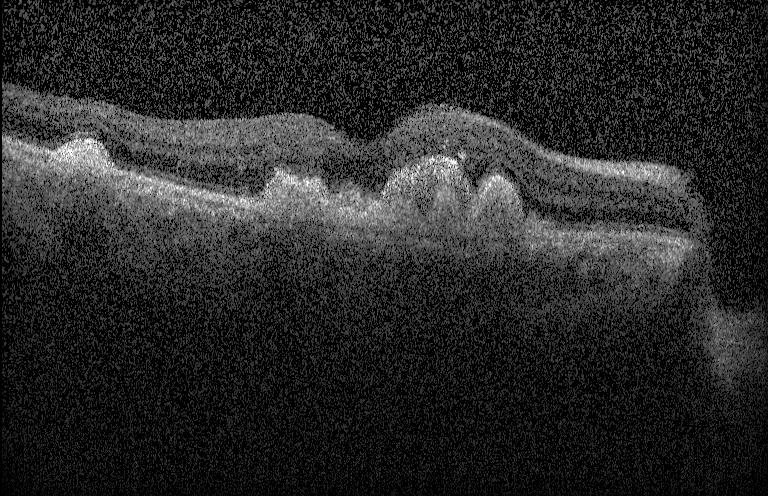
Finding: sub-RPE drusenoid deposits.